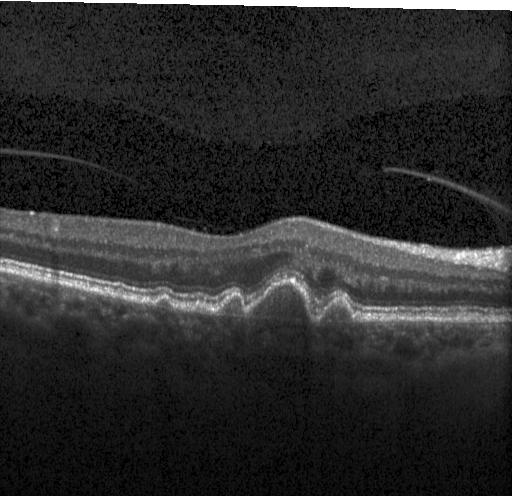
SD-OCT; OCT B-scan; acquired on a Heidelberg Spectralis; macular scan — Impression: choroidal neovascularization.